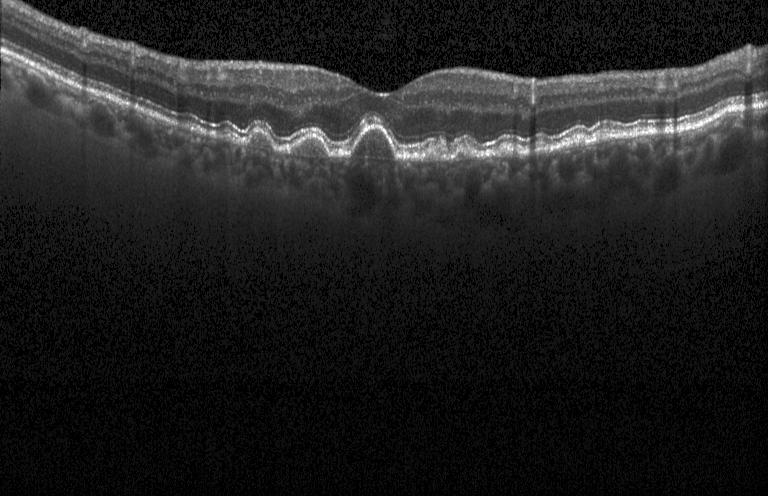 OCT line scan · spectral-domain OCT — Macular OCT: drusen.